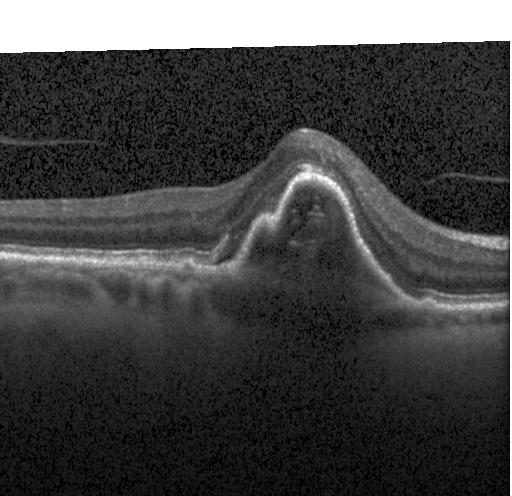
Optical coherence tomography B-scan — Assessment: CNV.